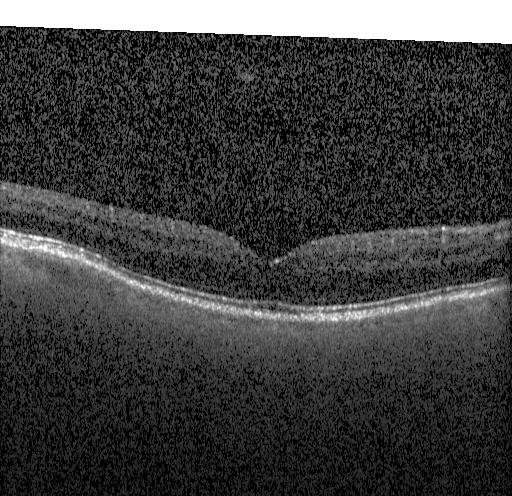 Retinal OCT cross-section.
Assessment: no choroidal neovascularization, no diabetic macular edema, and no drusen.